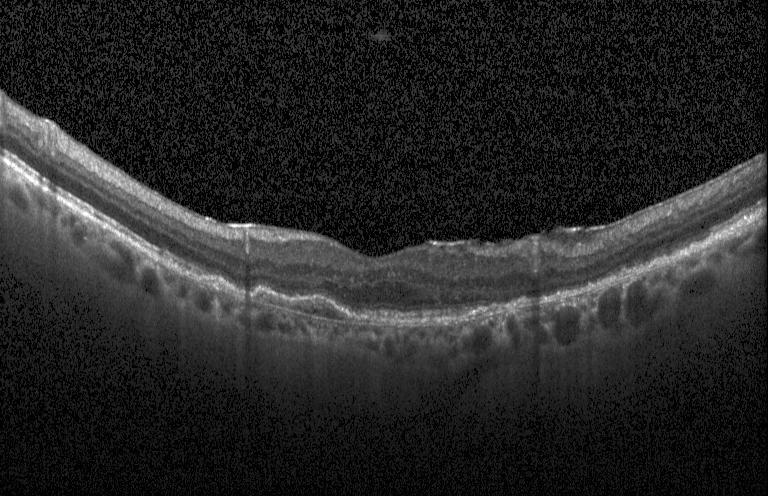 Fovea-centered. Acquired on a Heidelberg Spectralis. OCT line scan. Impression: choroidal neovascularization (CNV).